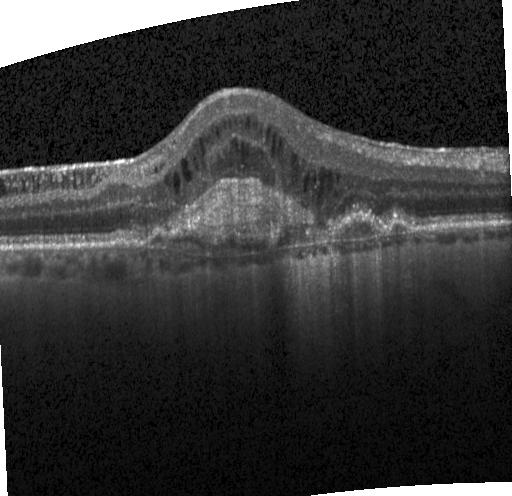 Optical coherence tomography B-scan.
OCT finding: choroidal neovascularization (CNV).